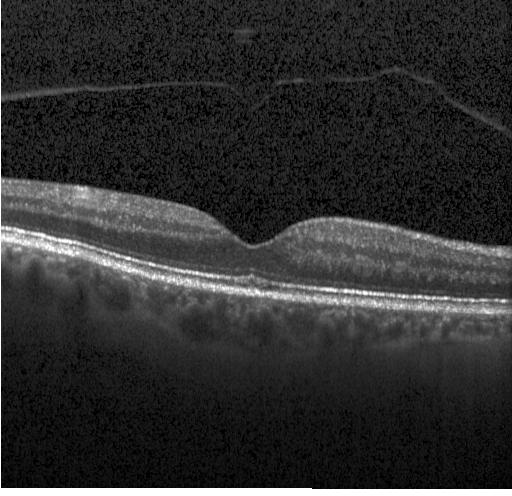 OCT B-scan — Impression: no evidence of choroidal neovascularization, diabetic macular edema, or drusen.